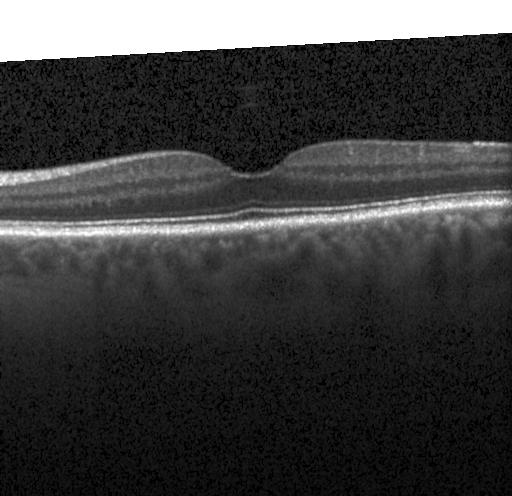 SD-OCT, OCT B-scan
The scan shows neither choroidal neovascularization, diabetic macular edema, nor drusen.